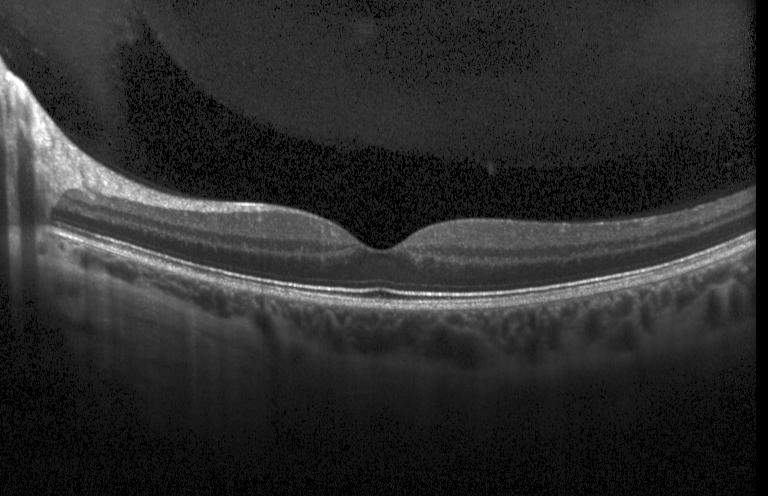 Through the macula, optical coherence tomography B-scan, instrument: Heidelberg Spectralis, spectral-domain optical coherence tomography — Impression: neither choroidal neovascularization, diabetic macular edema, nor drusen.